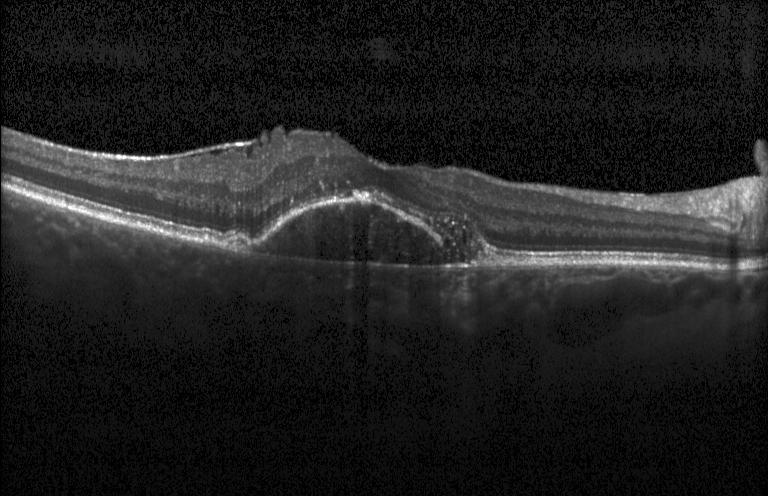
Optical coherence tomography scan. SD-OCT.
Finding: CNV.